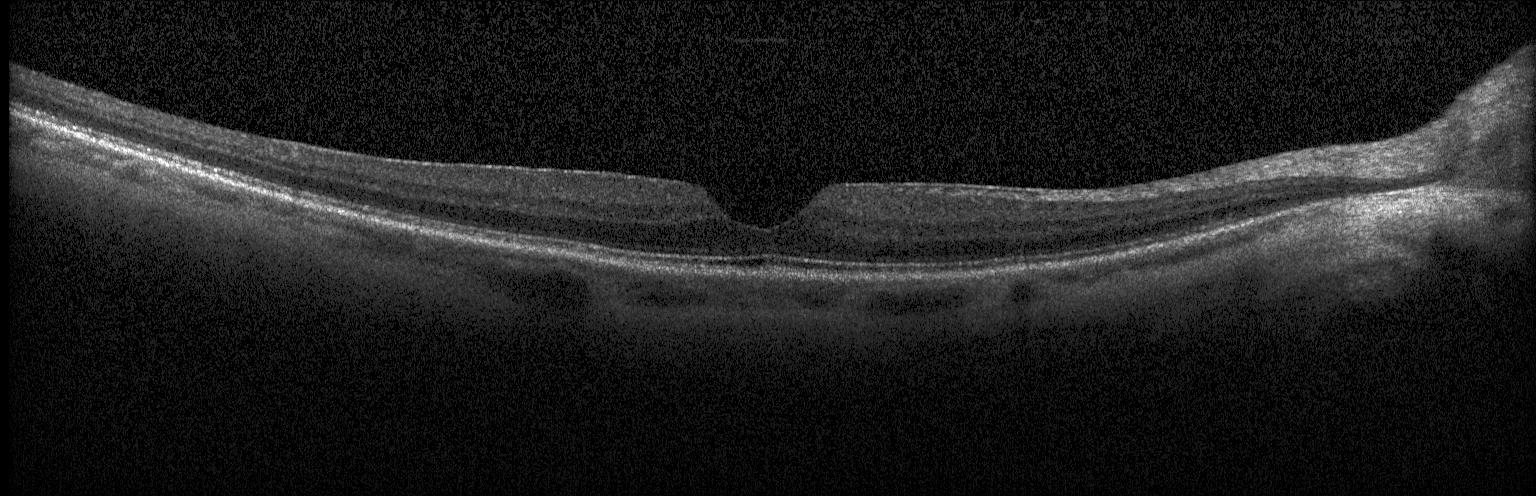
OCT line scan · SD-OCT · acquired on a Heidelberg Spectralis — The scan shows no evidence of choroidal neovascularization, diabetic macular edema, or drusen.